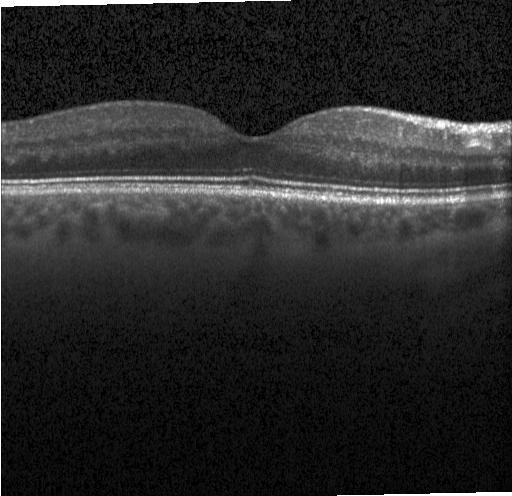
The scan shows no choroidal neovascularization, diabetic macular edema, or drusen.